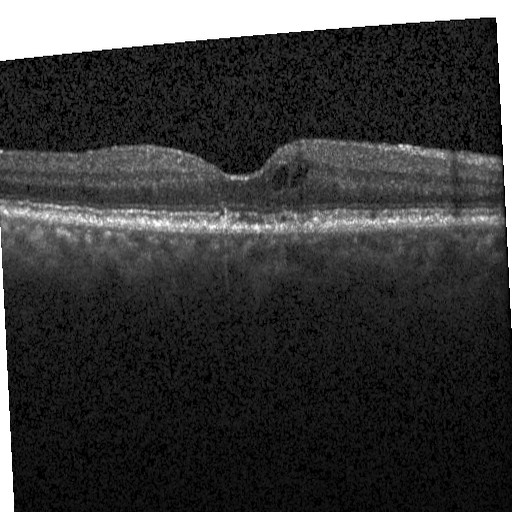

The scan shows diabetic macular edema.